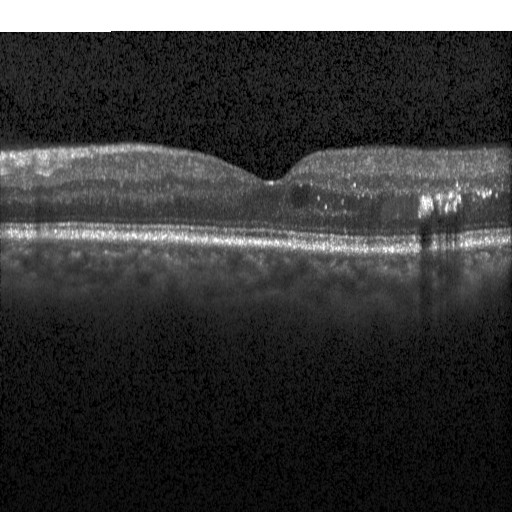

Optical coherence tomography B-scan
Diagnosis: diabetic macular edema (DME).